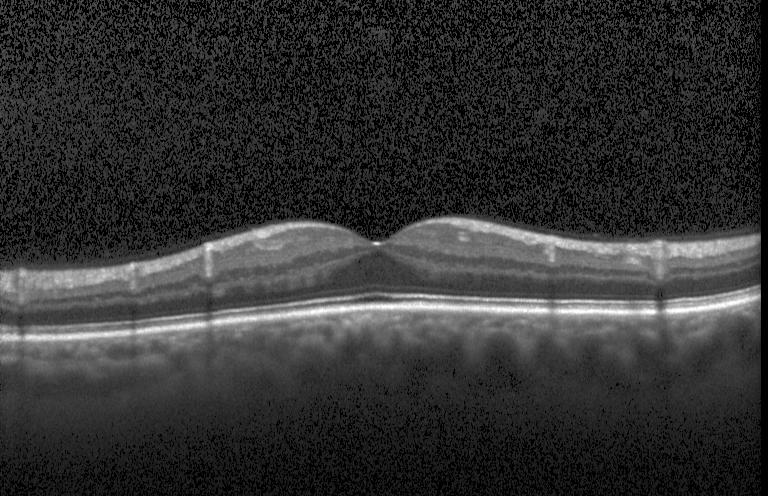

OCT finding: no evidence of choroidal neovascularization, diabetic macular edema, or drusen.